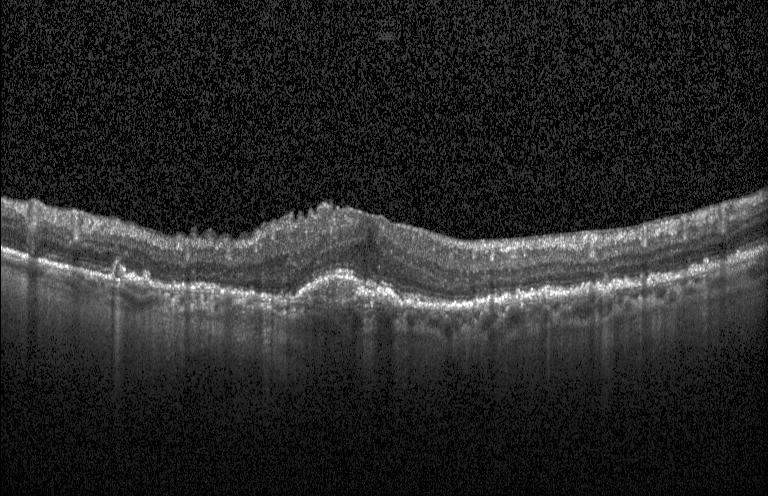 Dx: choroidal neovascularization.